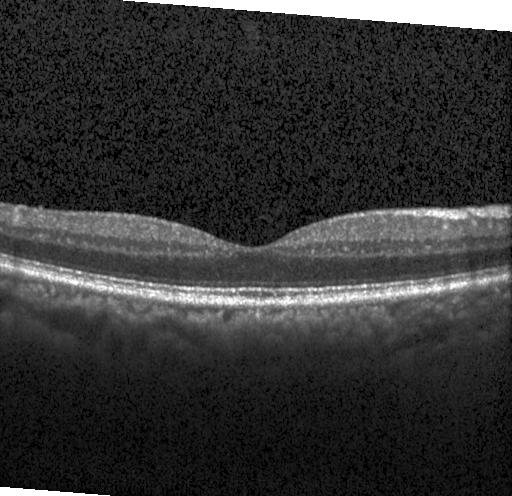

Diagnosis: no evidence of CNV, DME, or drusen.